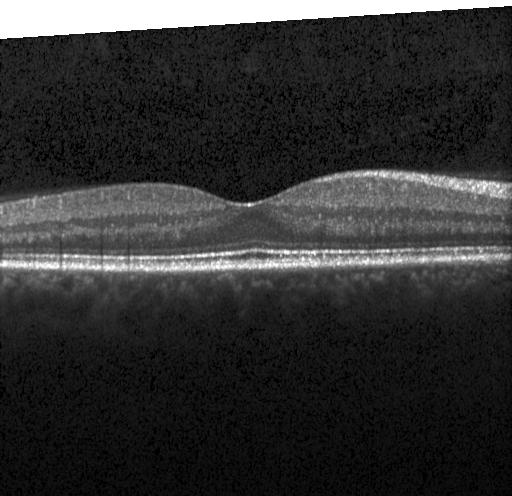
OCT line scan.
Assessment: neither choroidal neovascularization, diabetic macular edema, nor drusen.